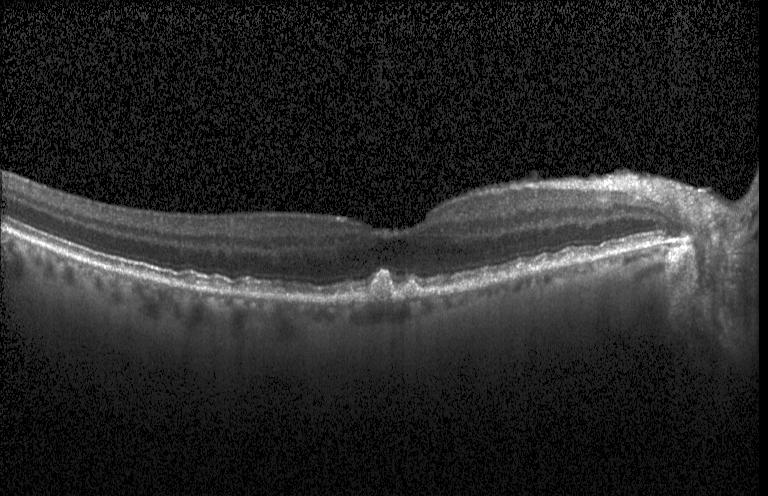
Instrument: Heidelberg Spectralis. Retinal OCT cross-section.
Impression: multiple drusen.